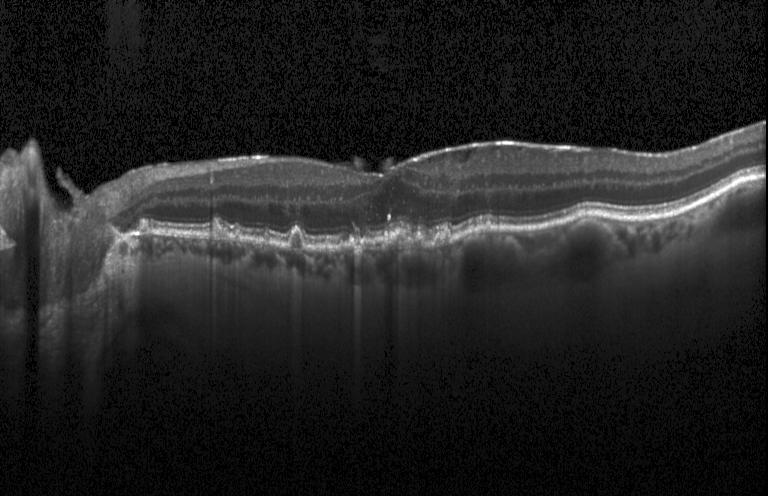

Acquired on a Heidelberg Spectralis, OCT B-scan — Finding: drusen.